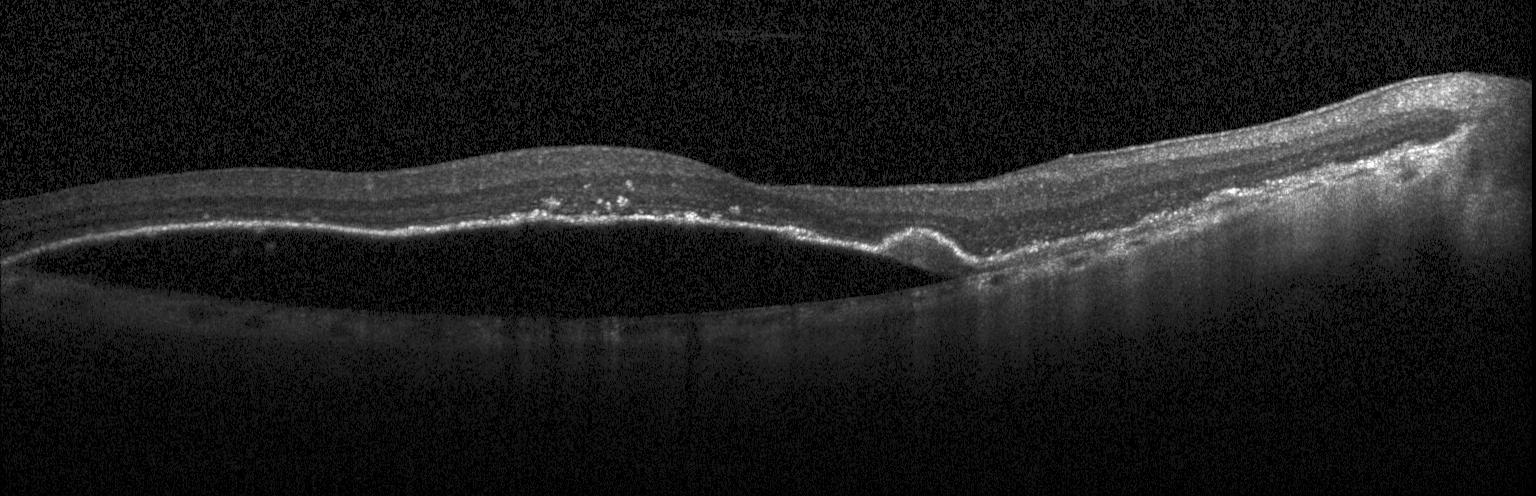

Retinal OCT B-scan.
Impression: a choroidal neovascular membrane.